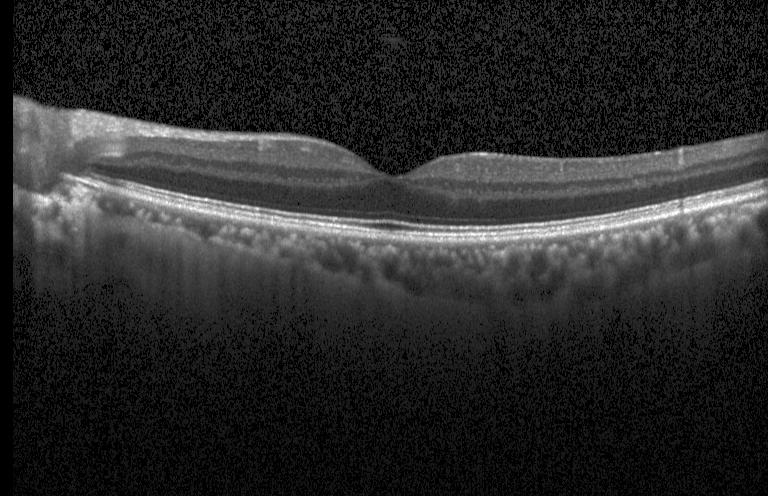
Diagnosis: neither CNV, DME, nor drusen.